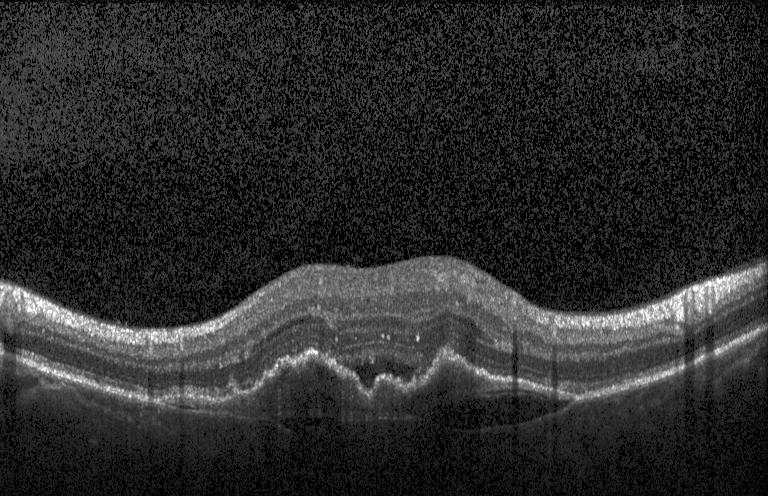
Fovea-centered, Heidelberg Spectralis OCT system, retinal OCT cross-section.
Impression: a choroidal neovascular membrane.